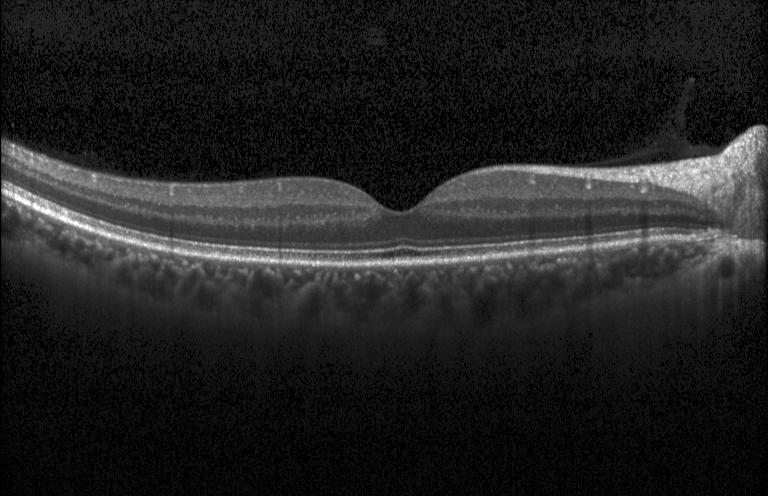 Optical coherence tomography B-scan. Diagnosis: no choroidal neovascularization, diabetic macular edema, or drusen.